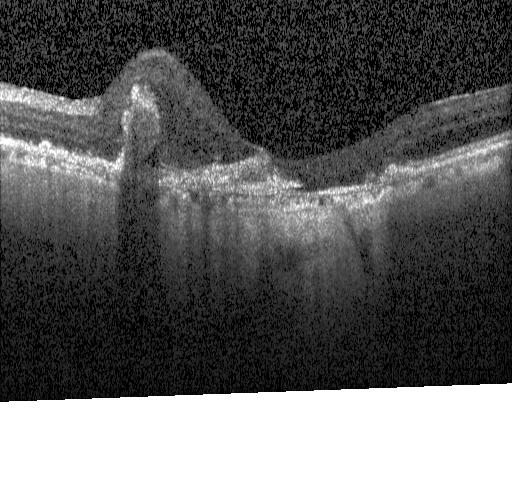
Finding: choroidal neovascularization (CNV).